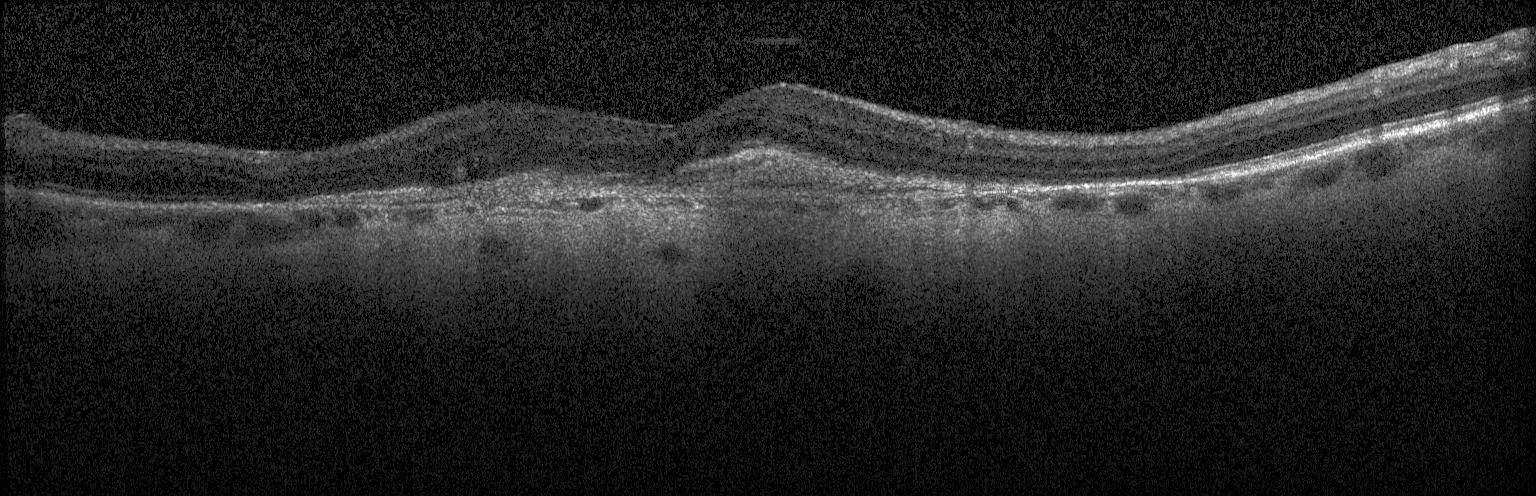 OCT finding: CNV.